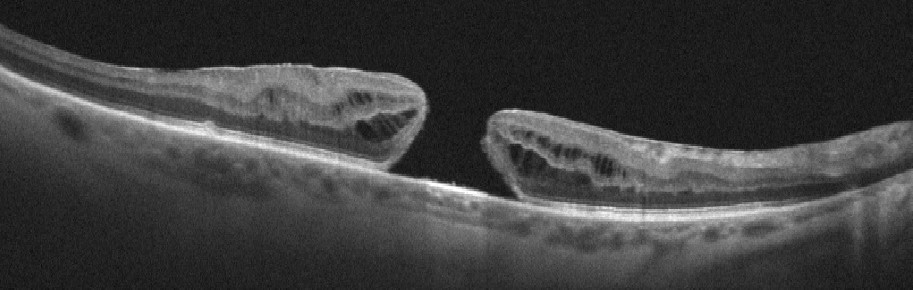

Retinal OCT B-scan. Instrument: Optovue Avanti RTVue XR.
Diagnosis: vitreomacular interface disease (VID).